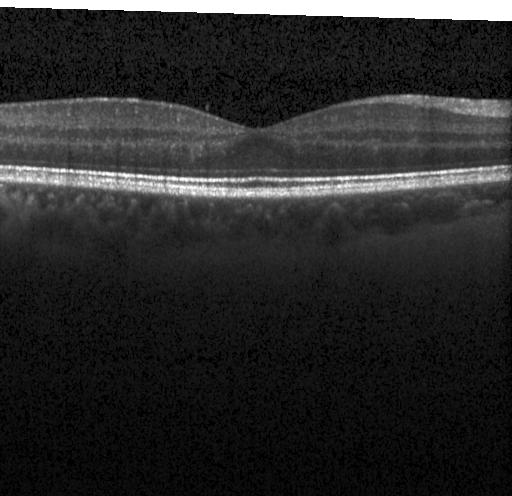
Assessment: no choroidal neovascularization, diabetic macular edema, or drusen.